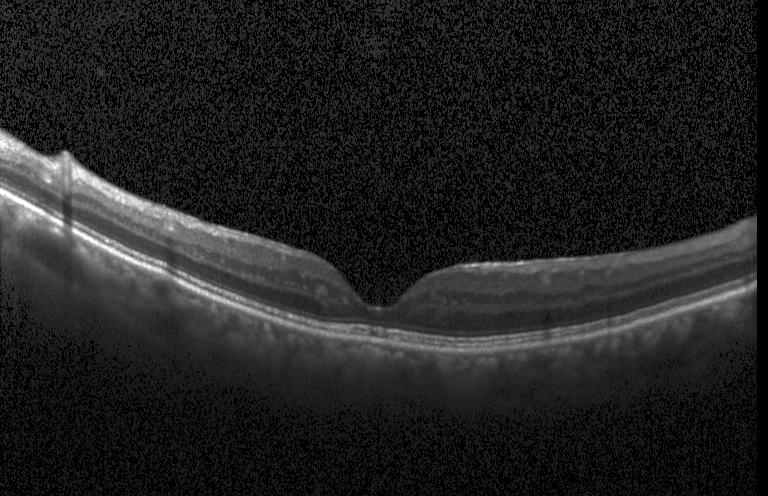 OCT finding: no choroidal neovascularization, diabetic macular edema, or drusen.